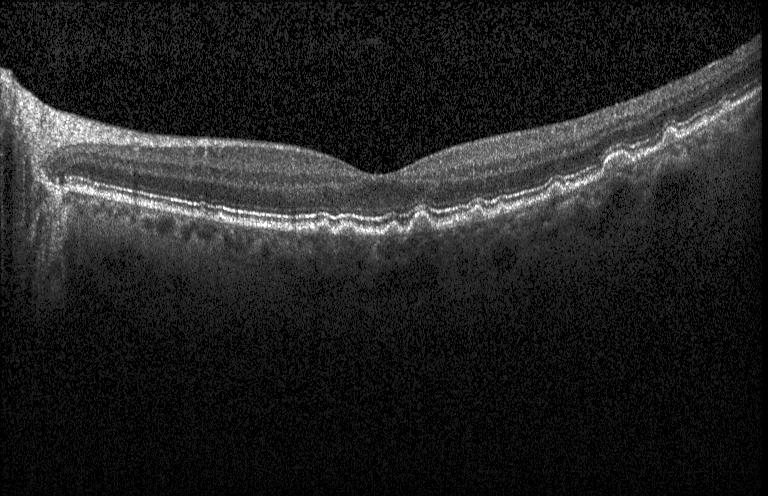 Finding: drusen.